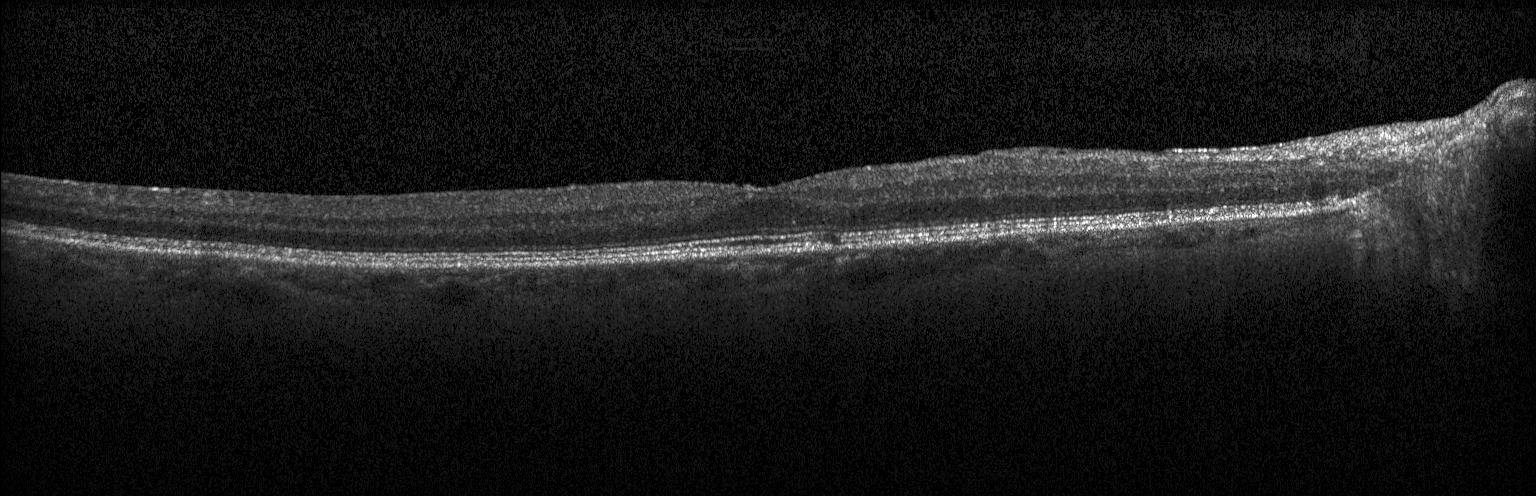

SD-OCT, fovea-centered, optical coherence tomography B-scan
No choroidal neovascularization, diabetic macular edema, or drusen.